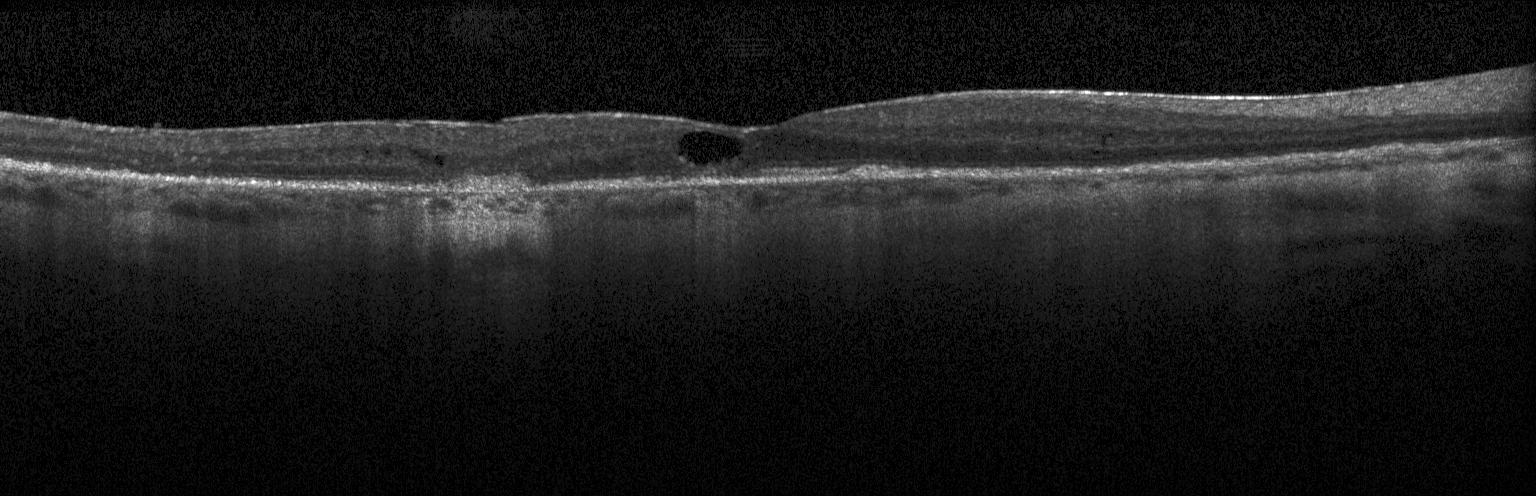 Optical coherence tomography B-scan · spectral-domain optical coherence tomography — Choroidal neovascularization (CNV).